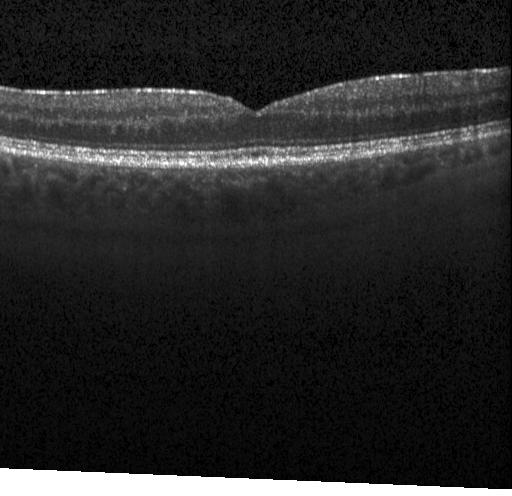

OCT finding: neither CNV, DME, nor drusen.